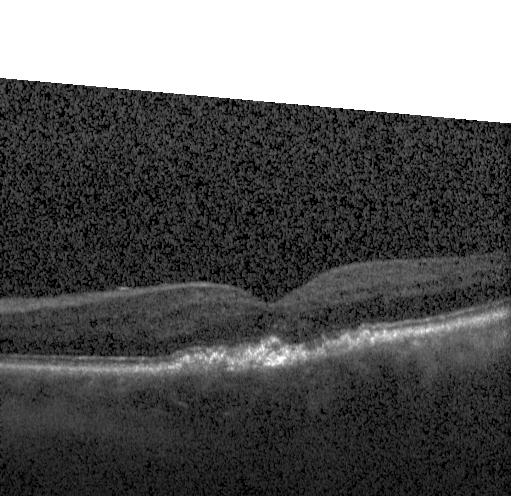

Optical coherence tomography scan
Diagnosis: CNV.